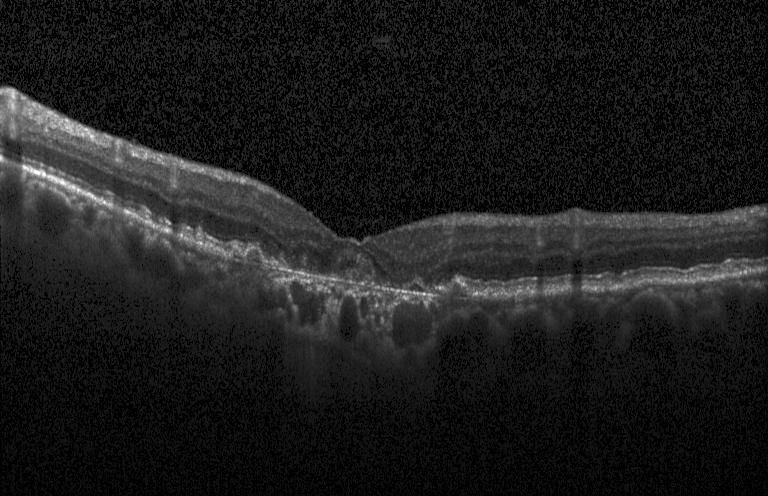 Macular OCT demonstrating a choroidal neovascular membrane.